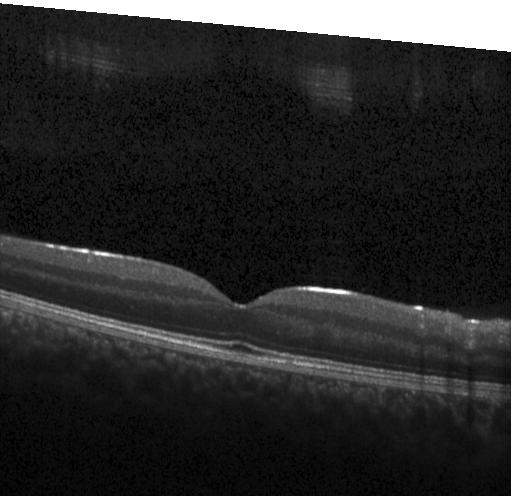 Optical coherence tomography B-scan. Impression: no evidence of CNV, DME, or drusen.